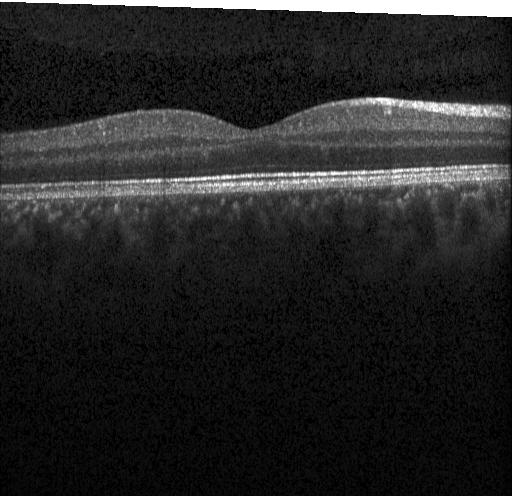 OCT scan showing no evidence of CNV, DME, or drusen.